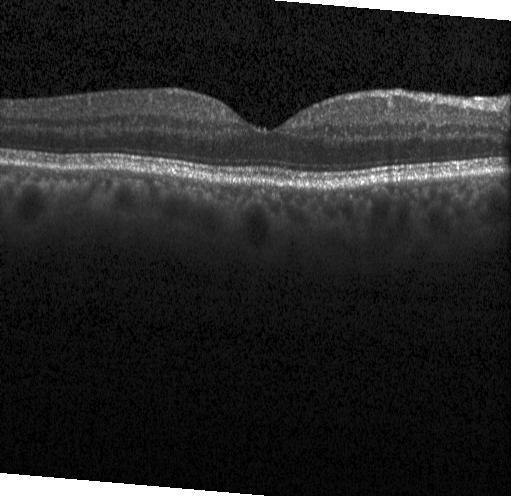
Assessment: no choroidal neovascularization, no diabetic macular edema, and no drusen.